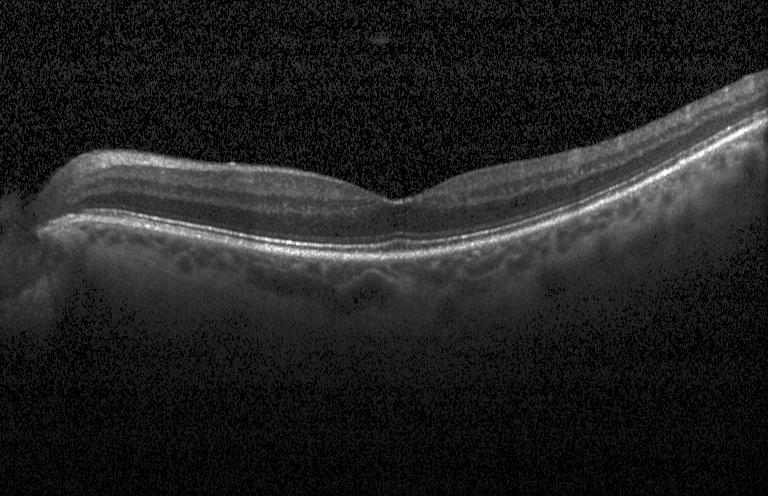 OCT B-scan — The scan shows no CNV, no DME, and no drusen.